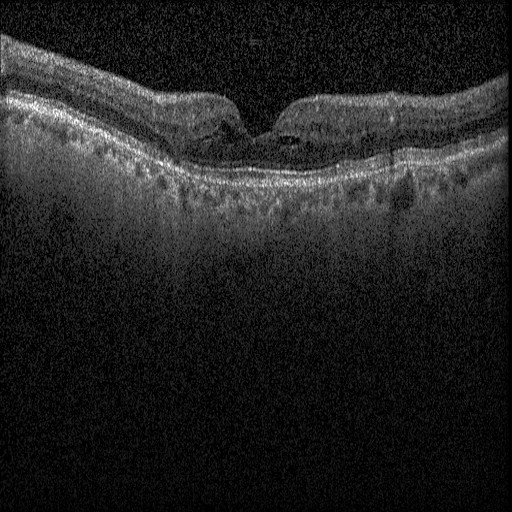

Macular OCT demonstrating diabetic macular edema.